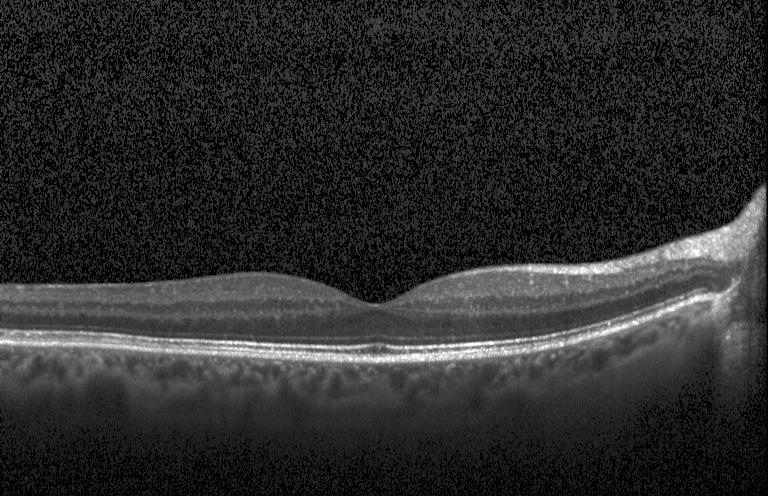 Centered on the fovea; retinal OCT B-scan; acquired on a Heidelberg Spectralis; spectral-domain optical coherence tomography
Dx: neither choroidal neovascularization, diabetic macular edema, nor drusen.